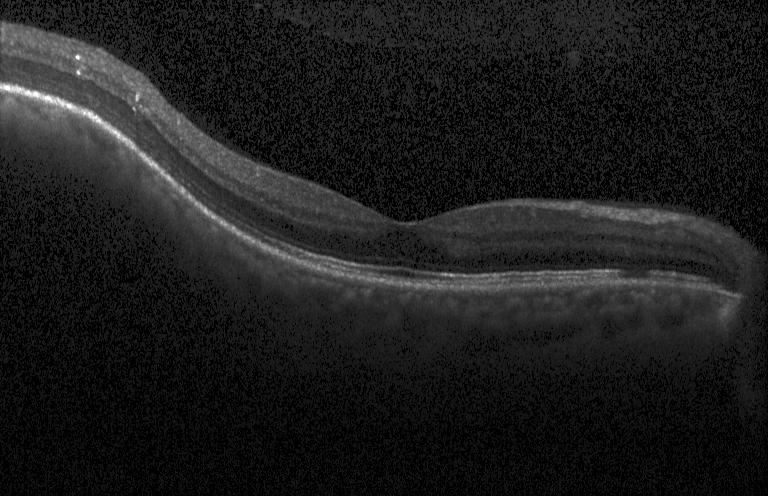
Spectral-domain optical coherence tomography, acquired on a Heidelberg Spectralis, OCT B-scan — Impression: no evidence of choroidal neovascularization, diabetic macular edema, or drusen.